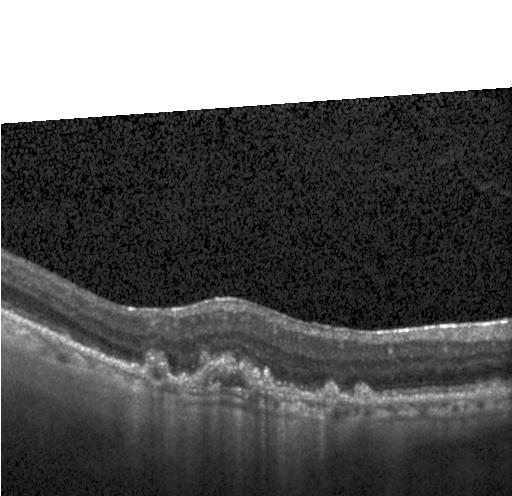

Spectral-domain OCT, optical coherence tomography scan. Finding: CNV.